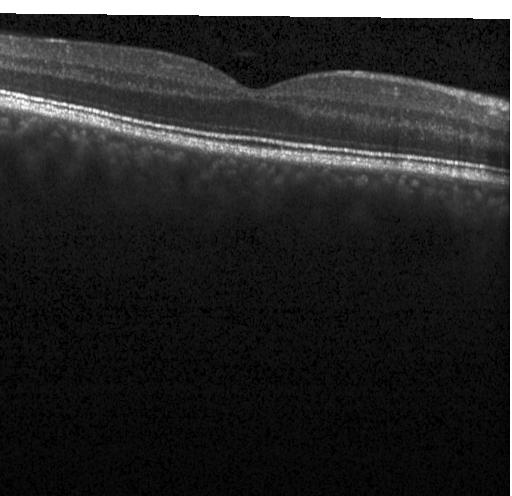 Retinal OCT cross-section. Centered on the fovea. Spectral-domain optical coherence tomography. Instrument: Heidelberg Spectralis — Finding: no evidence of choroidal neovascularization, diabetic macular edema, or drusen.